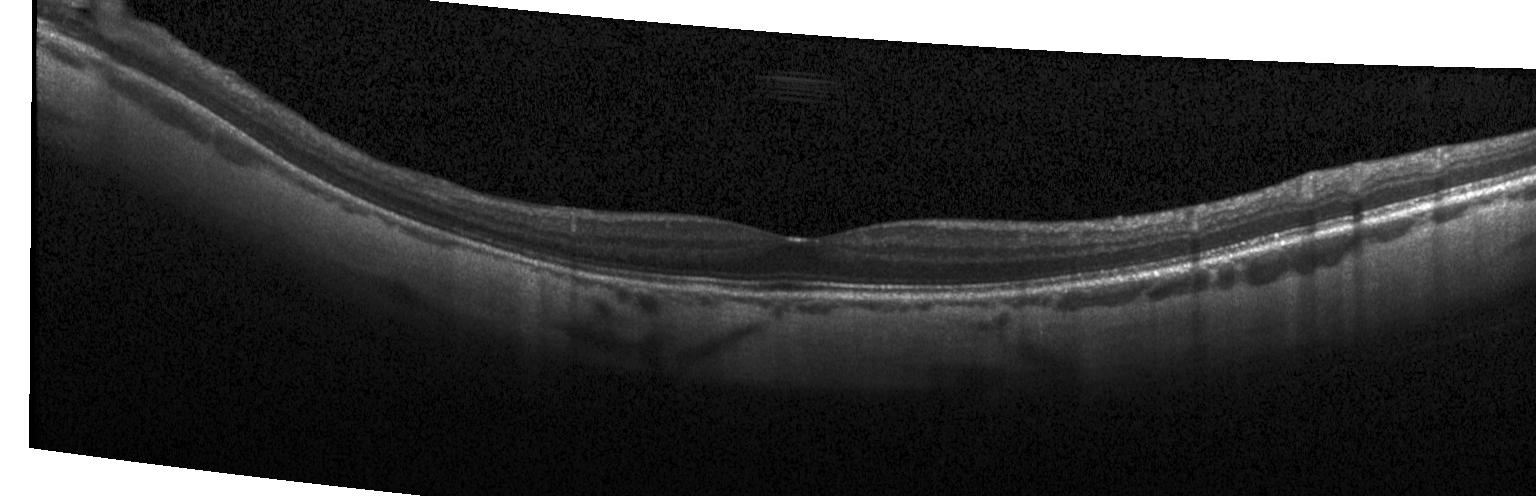 OCT finding: neither CNV, DME, nor drusen.